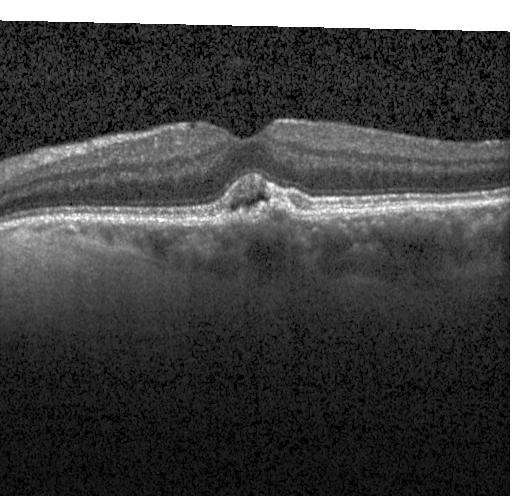

SD-OCT, optical coherence tomography scan, fovea-centered — Impression: a choroidal neovascular membrane.